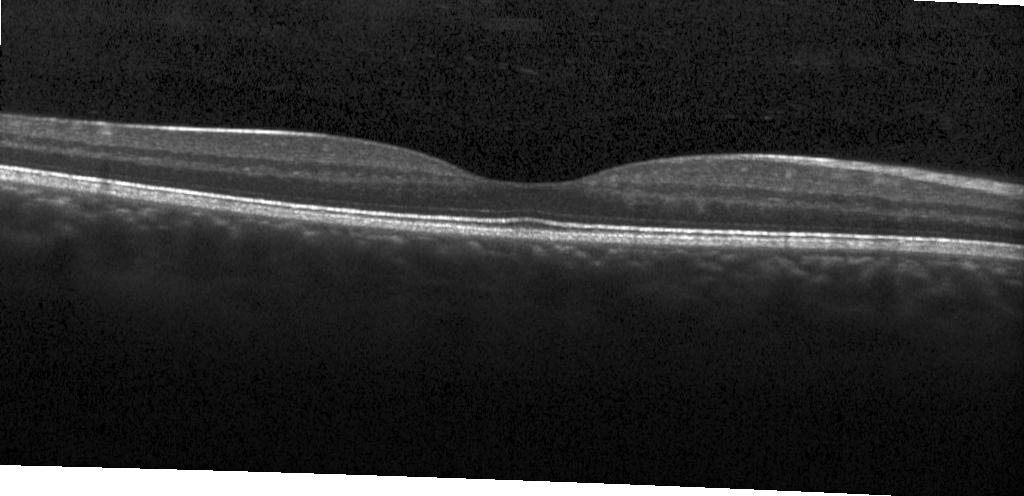 Centered on the fovea, spectral-domain optical coherence tomography, optical coherence tomography B-scan.
Impression: neither choroidal neovascularization, diabetic macular edema, nor drusen.